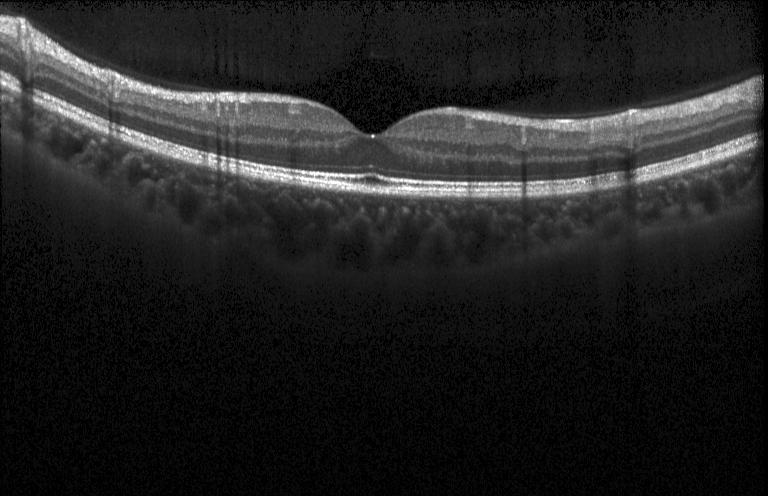
Retinal OCT B-scan
Macular OCT: no choroidal neovascularization, diabetic macular edema, or drusen.